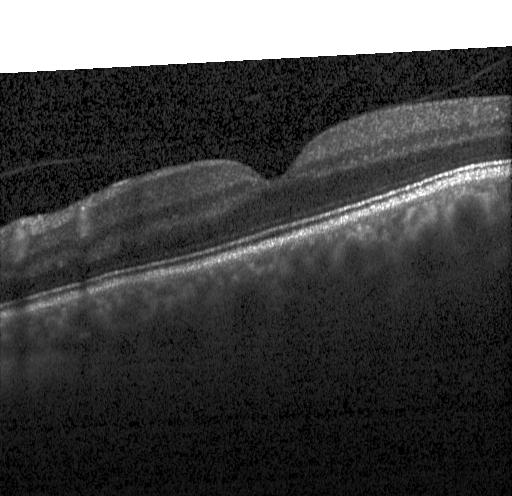
Retinal OCT cross-section
Diagnosis: neither CNV, DME, nor drusen.